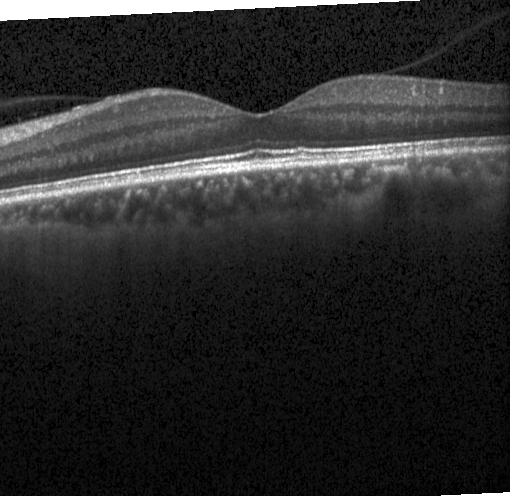

Optical coherence tomography B-scan · SD-OCT · instrument: Heidelberg Spectralis · centered on the fovea. Diagnosis: multiple drusen.